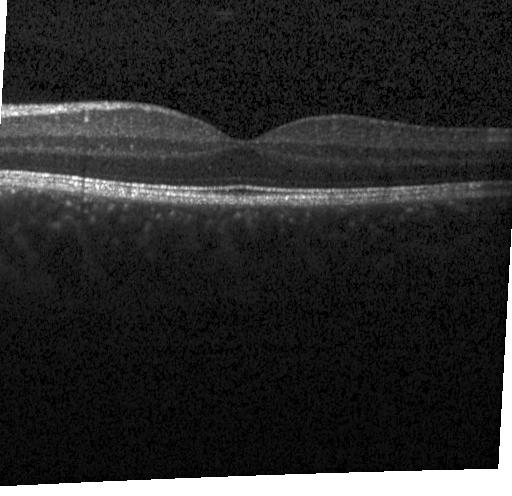 SD-OCT. Centered on the fovea. OCT B-scan. Heidelberg Spectralis OCT system. Diagnosis: no evidence of choroidal neovascularization, diabetic macular edema, or drusen.